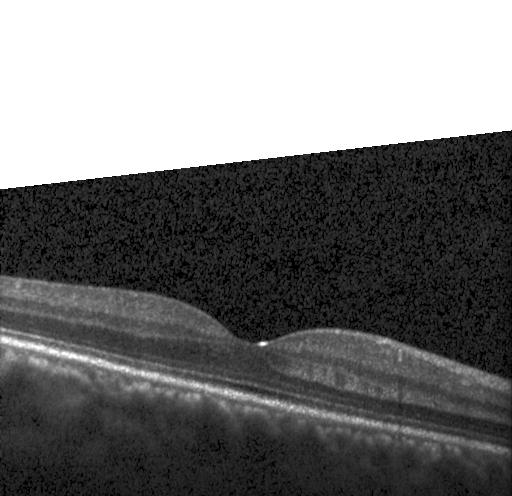
Macular OCT: no choroidal neovascularization, diabetic macular edema, or drusen.